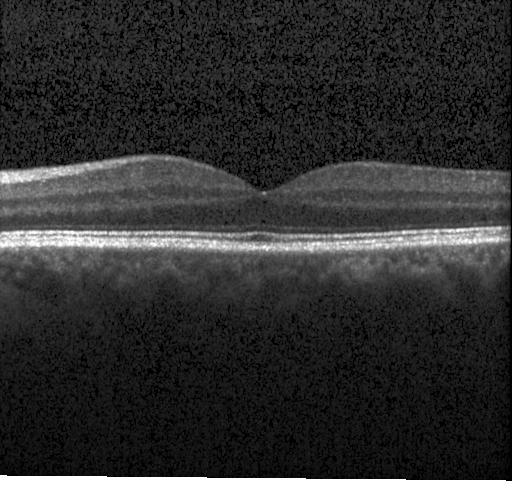

OCT B-scan, acquired on a Heidelberg Spectralis, through the macula
Impression: no choroidal neovascularization, no diabetic macular edema, and no drusen.